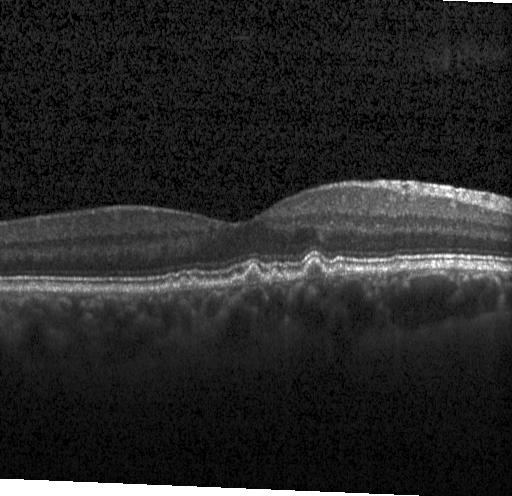
Optical coherence tomography scan, Heidelberg Spectralis OCT system — Impression: multiple drusen.